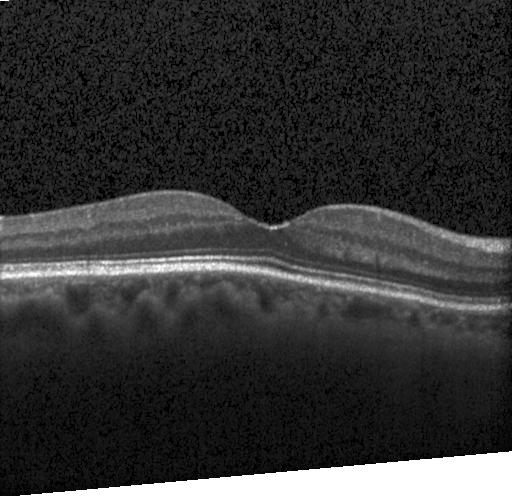
OCT scan showing no choroidal neovascularization, diabetic macular edema, or drusen.